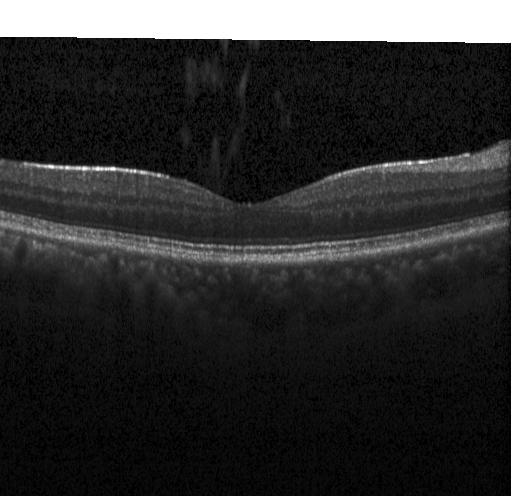

Retinal OCT B-scan; Heidelberg Spectralis OCT system; through the macula.
Finding: no choroidal neovascularization, no diabetic macular edema, and no drusen.